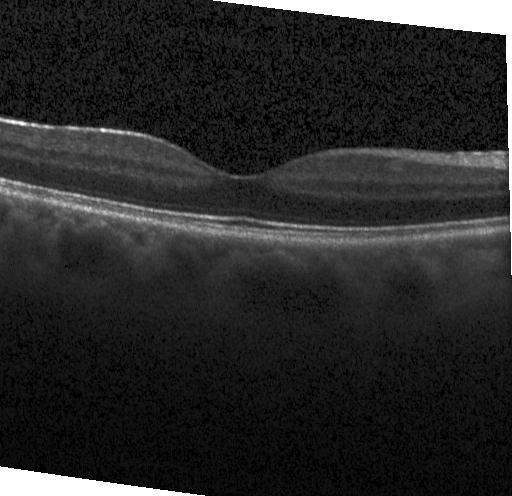
Finding: no evidence of choroidal neovascularization, diabetic macular edema, or drusen.